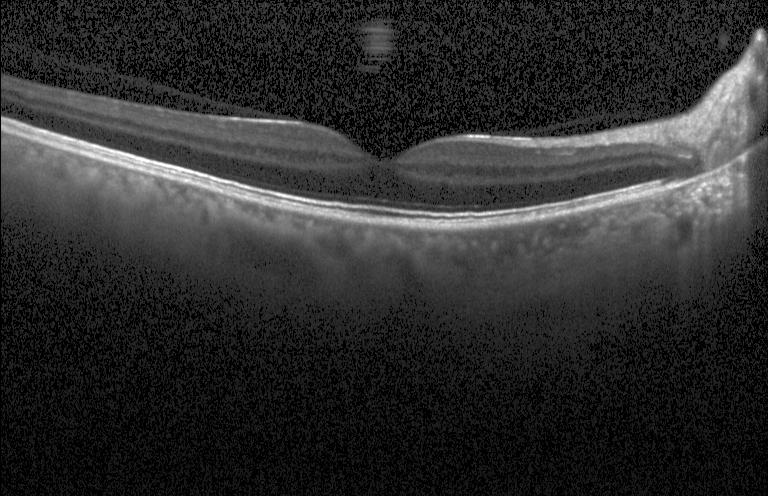 Impression: no choroidal neovascularization, no diabetic macular edema, and no drusen.